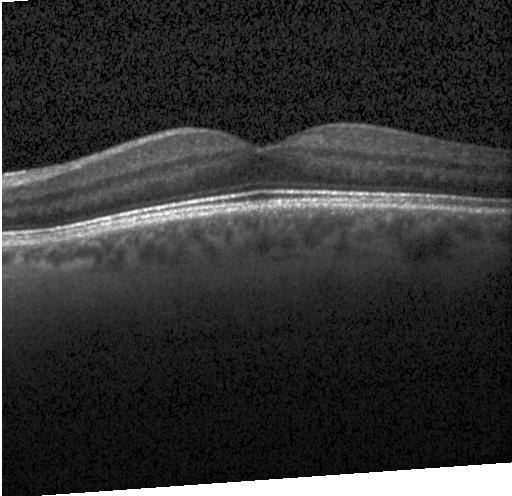

Spectral-domain OCT · Heidelberg Spectralis · macular scan · retinal OCT B-scan
Assessment: no evidence of choroidal neovascularization, diabetic macular edema, or drusen.